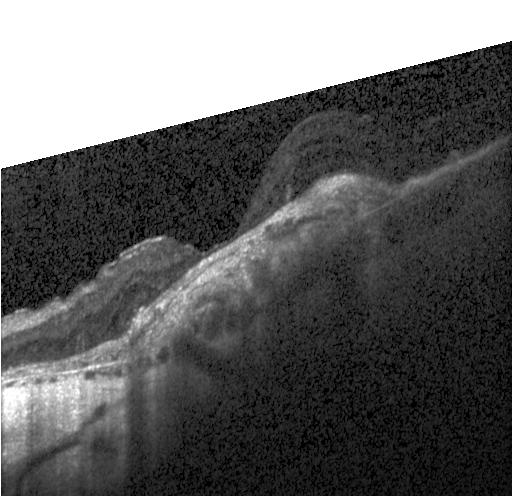
Heidelberg Spectralis, horizontal scan through the fovea, SD-OCT, optical coherence tomography B-scan.
Assessment: CNV.